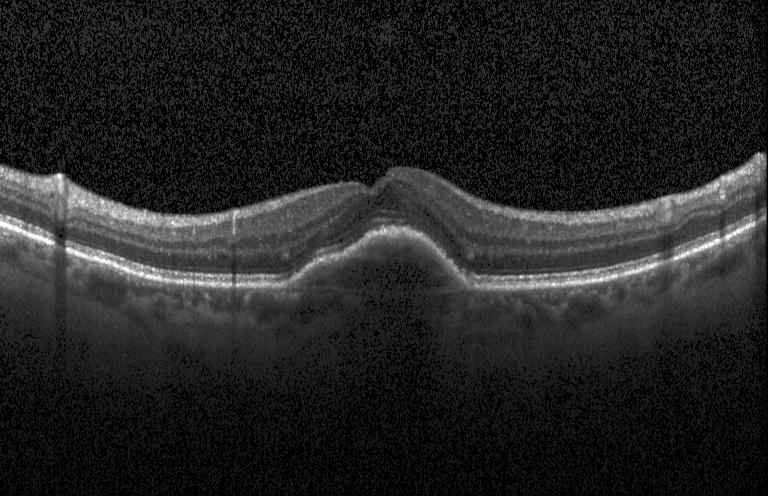

OCT B-scan
This B-scan demonstrates a choroidal neovascular membrane.